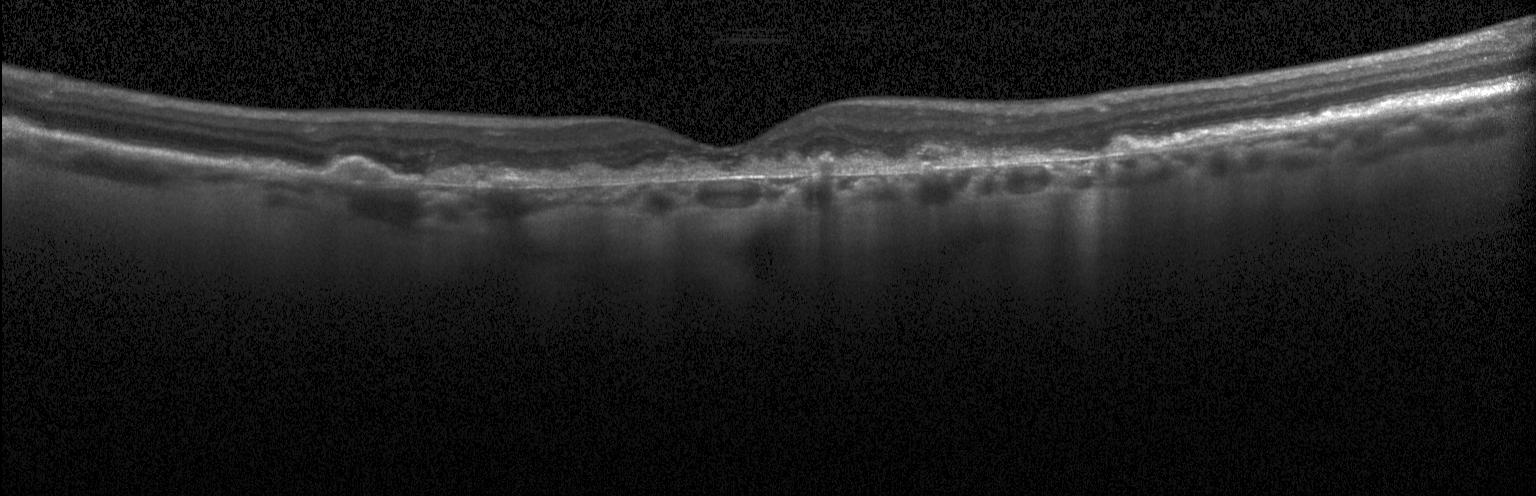

Acquired on a Heidelberg Spectralis · retinal OCT cross-section · fovea-centered. Impression: CNV.